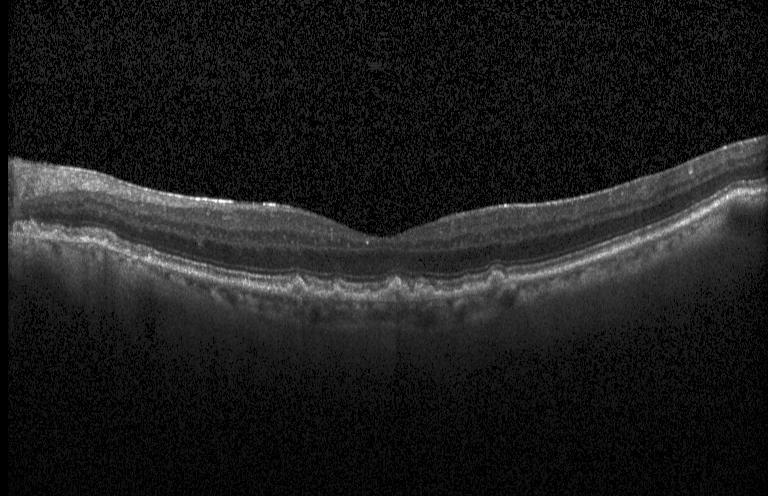
Finding: drusen.